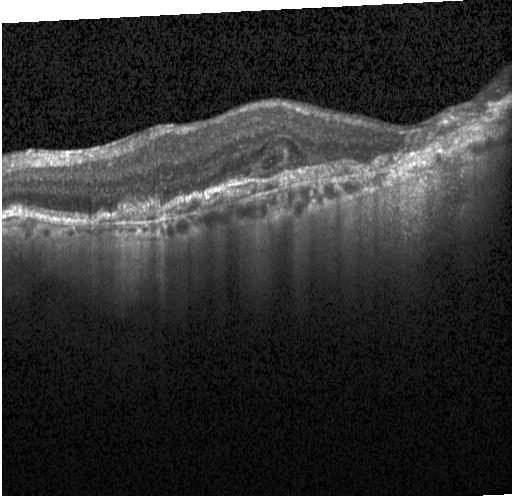

Heidelberg Spectralis, OCT B-scan, SD-OCT.
Impression: CNV.